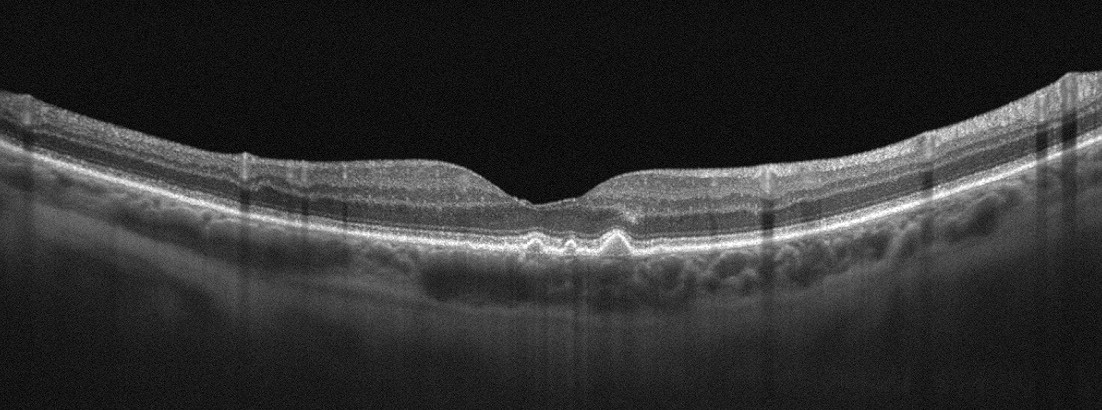

Instrument: Optovue Avanti RTVue XR · retinal OCT cross-section · fovea-centered.
Macular OCT: age-related macular degeneration.